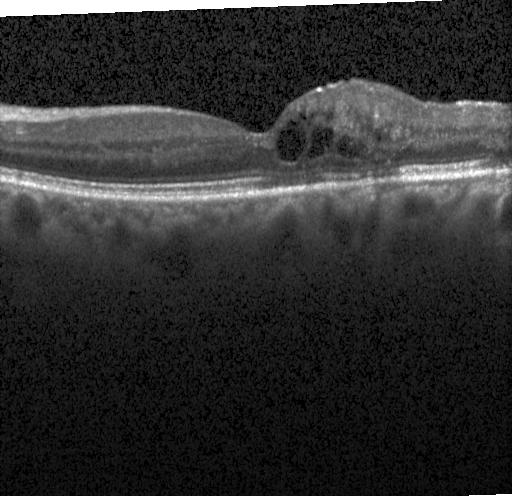

Heidelberg Spectralis; OCT line scan. This B-scan demonstrates diabetic macular edema.